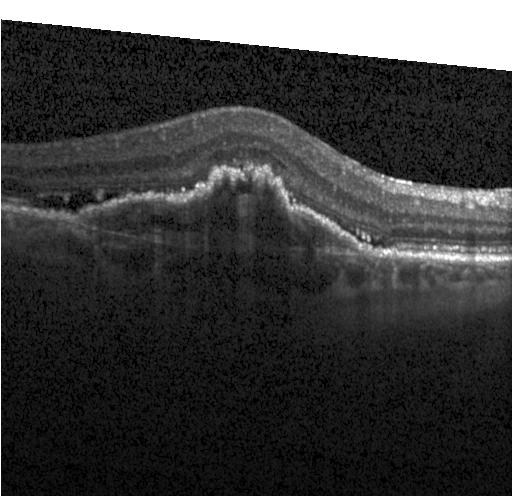

OCT finding: CNV.